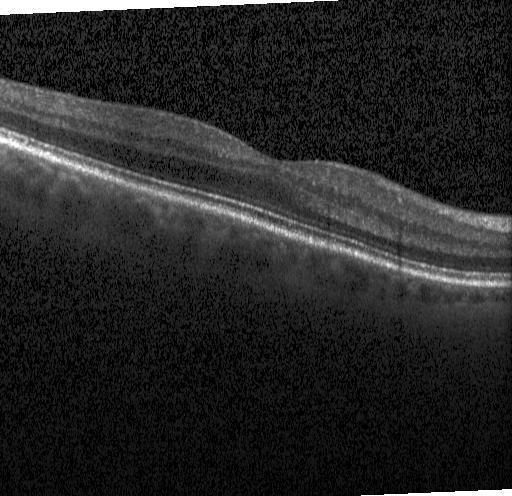

Finding: no evidence of choroidal neovascularization, diabetic macular edema, or drusen.